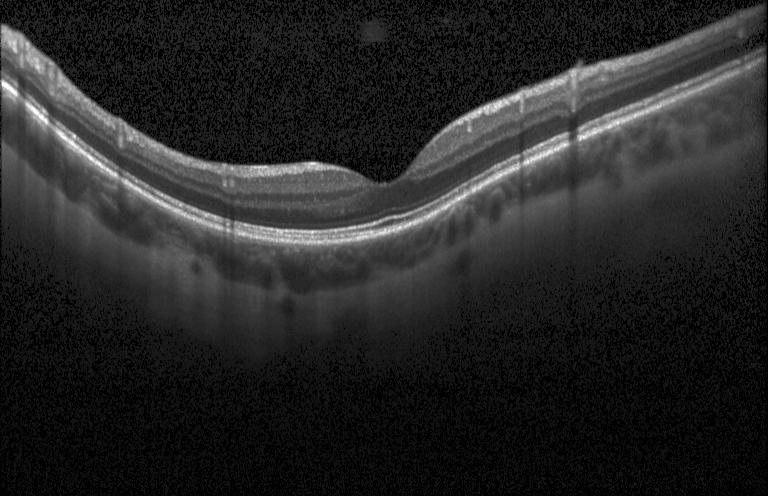

OCT finding: no choroidal neovascularization, no diabetic macular edema, and no drusen.